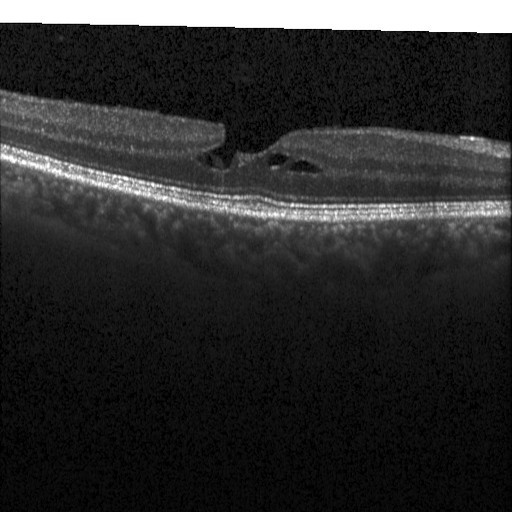

Spectral-domain OCT · acquired on a Heidelberg Spectralis · retinal OCT cross-section · through the macula — Diagnosis: DME.